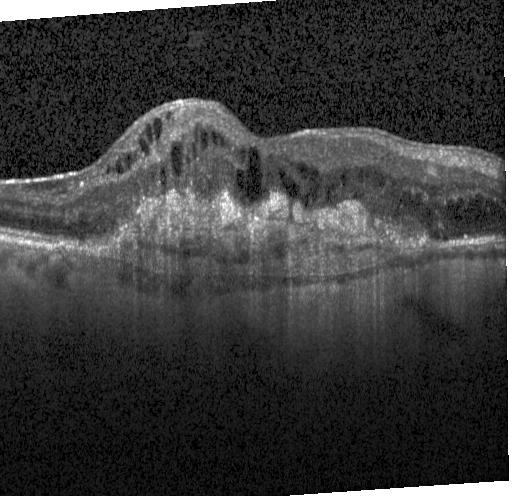 Macular OCT: choroidal neovascularization (CNV).